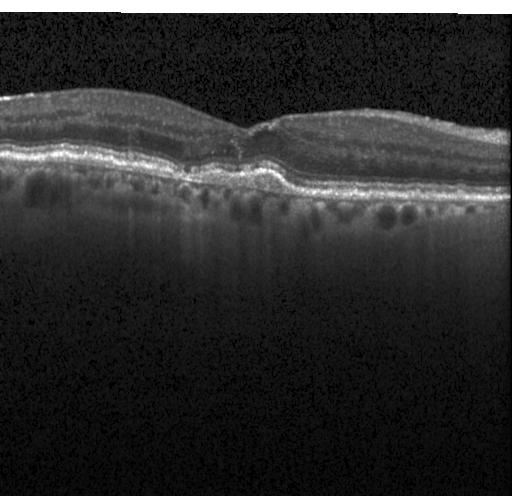 OCT finding: a choroidal neovascular membrane.